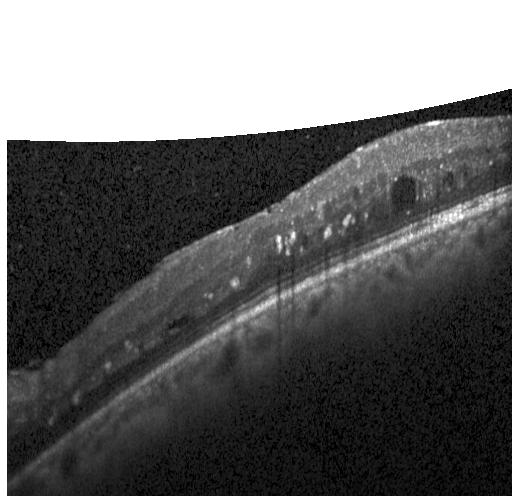 Macular scan · optical coherence tomography scan.
Diagnosis: DME.